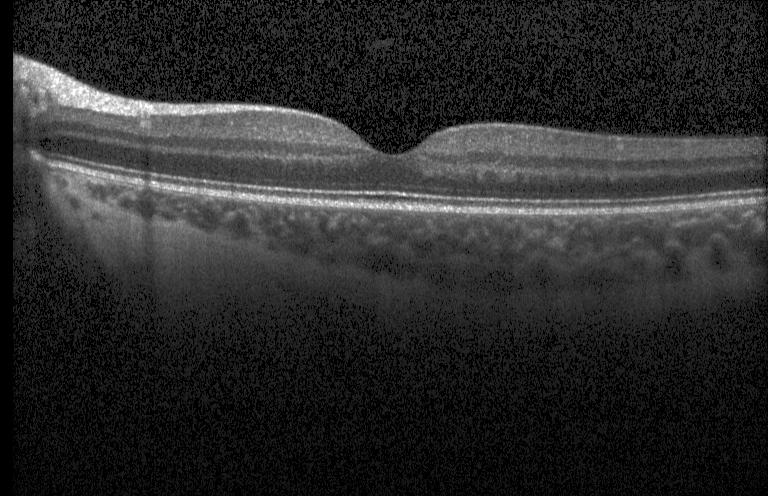

Optical coherence tomography scan · spectral-domain optical coherence tomography · through the macula — OCT finding: no CNV, DME, or drusen.